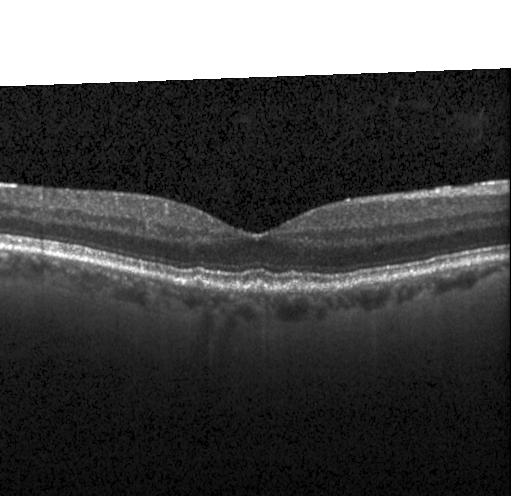 Spectral-domain OCT B-scan: multiple drusen.